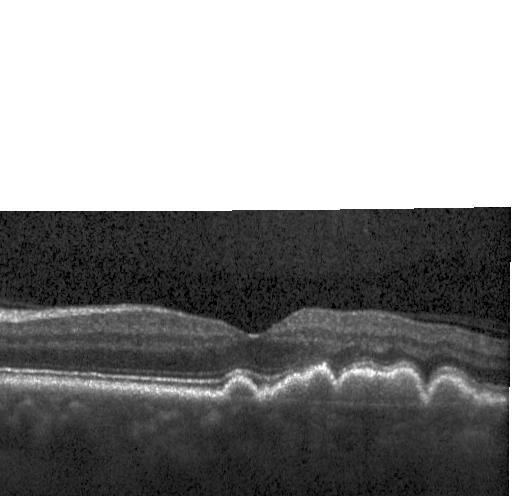
SD-OCT; fovea-centered; OCT line scan; instrument: Heidelberg Spectralis. Impression: drusen.